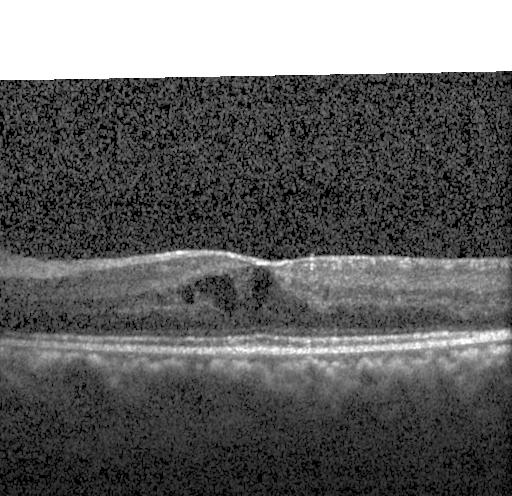
SD-OCT, instrument: Heidelberg Spectralis, centered on the fovea, retinal OCT cross-section
Finding: DME.